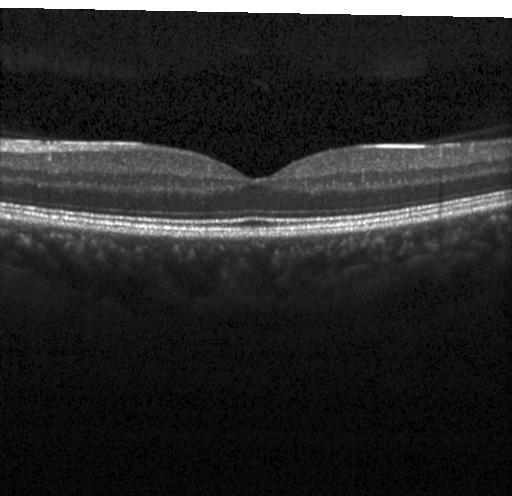
Dx: no CNV, DME, or drusen.